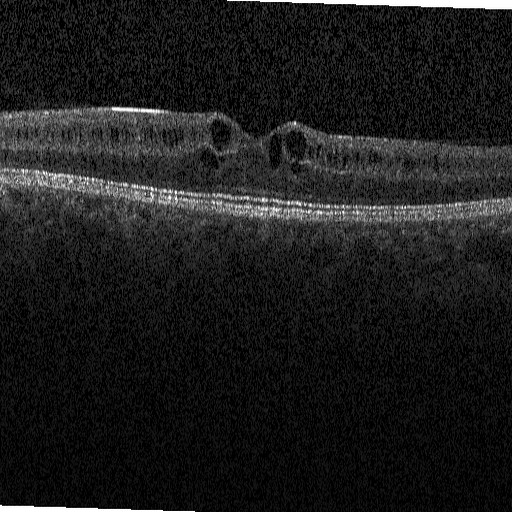
OCT B-scan — OCT finding: diabetic macular edema.